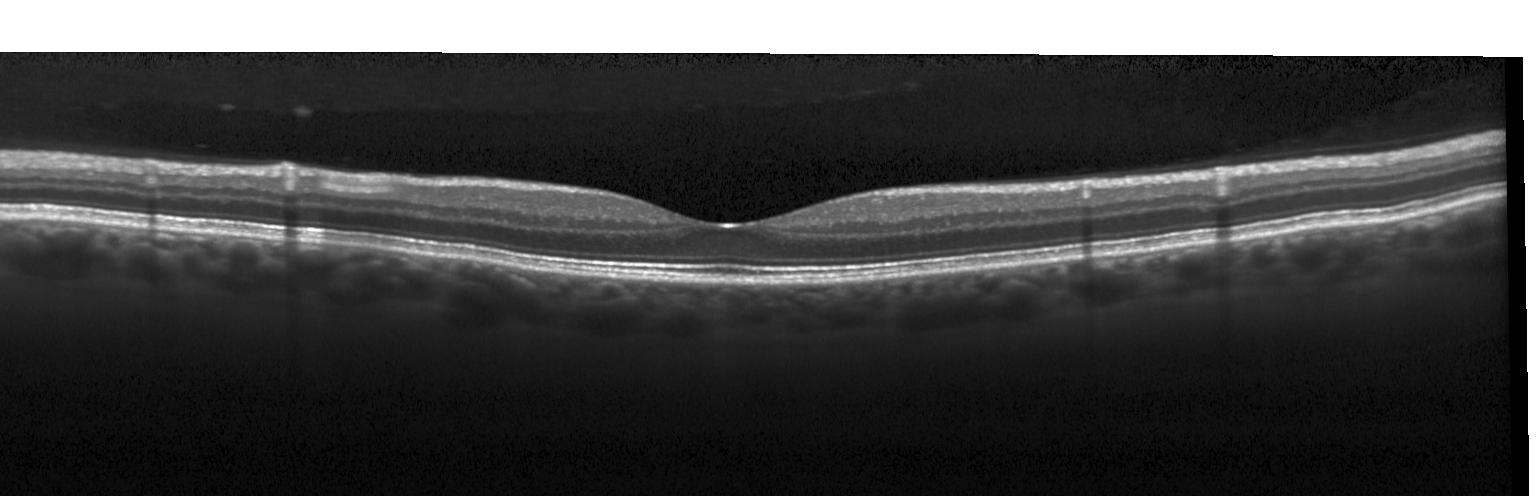 SD-OCT · OCT line scan — Diagnosis: no choroidal neovascularization, diabetic macular edema, or drusen.